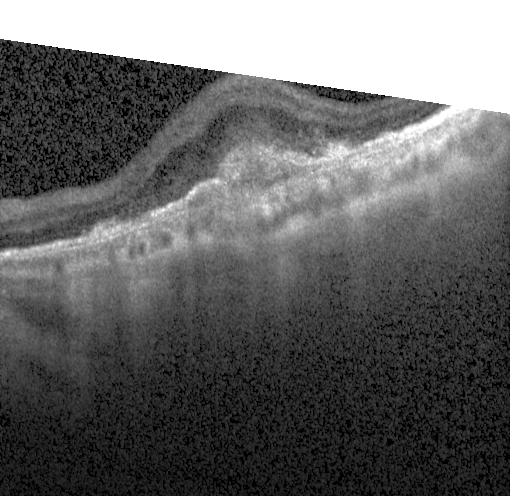
Assessment: a choroidal neovascular membrane.